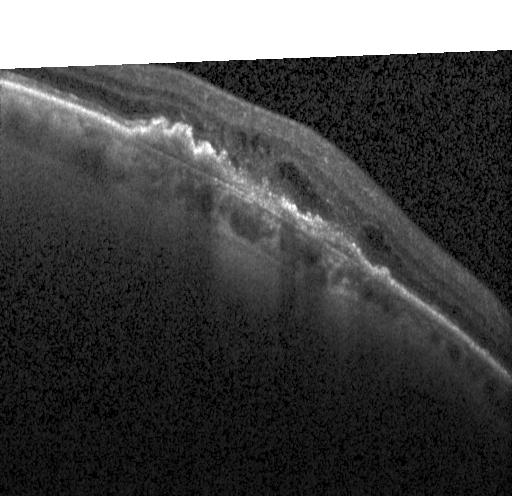
Spectral-domain optical coherence tomography · OCT B-scan · fovea-centered — Impression: a choroidal neovascular membrane.